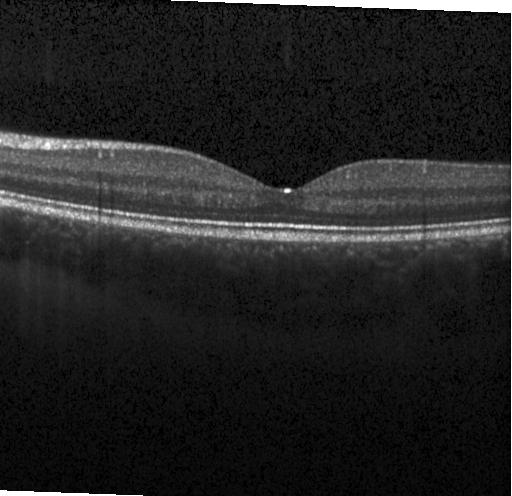

Spectral-domain OCT · optical coherence tomography B-scan.
OCT finding: no choroidal neovascularization, no diabetic macular edema, and no drusen.